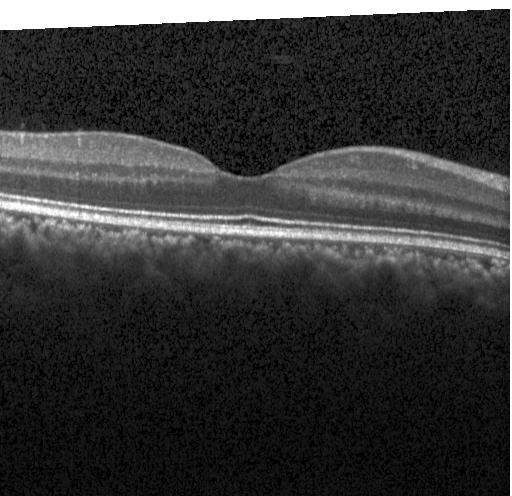
Macular OCT demonstrating no choroidal neovascularization, diabetic macular edema, or drusen.